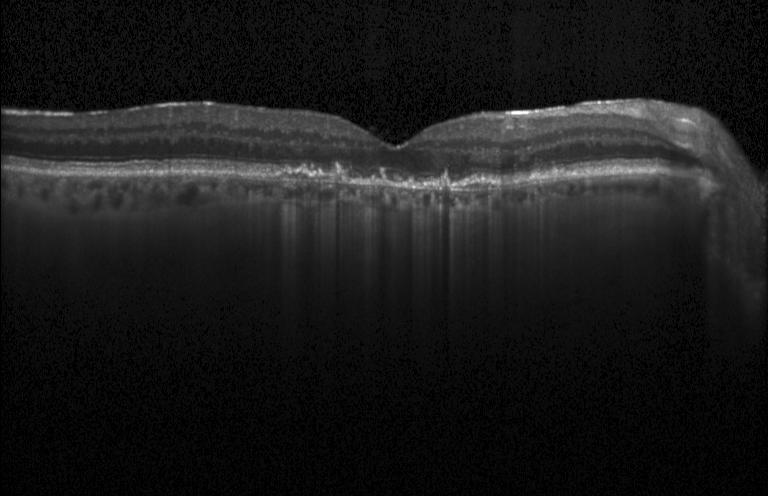 Horizontal scan through the fovea. Spectral-domain OCT. OCT B-scan
Dx: CNV.